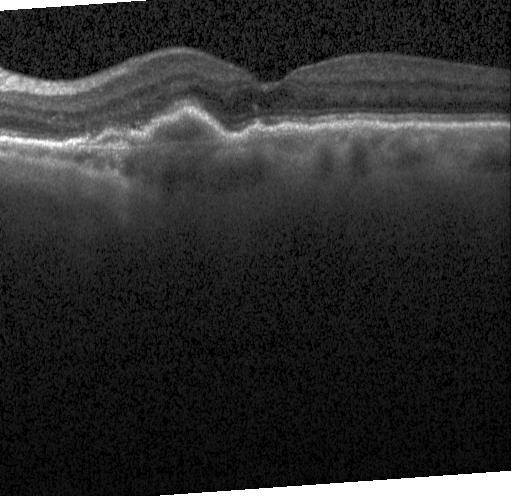 Spectral-domain OCT · retinal OCT cross-section · instrument: Heidelberg Spectralis
This B-scan demonstrates choroidal neovascularization.